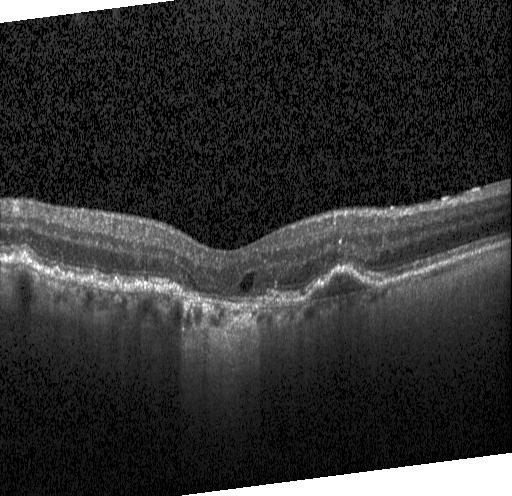
Retinal OCT B-scan · through the macula
Impression: a choroidal neovascular membrane.